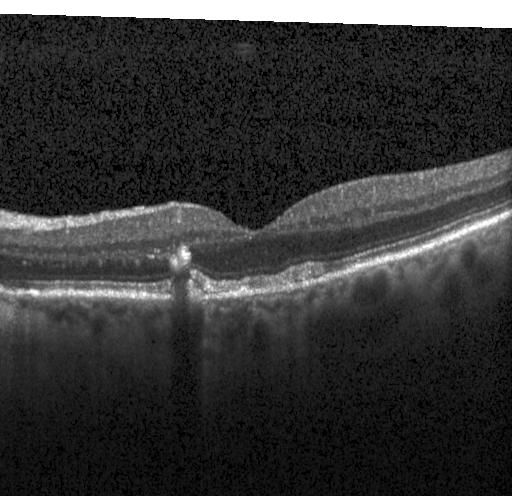

Optical coherence tomography scan · Heidelberg Spectralis OCT system. This B-scan demonstrates multiple drusen.